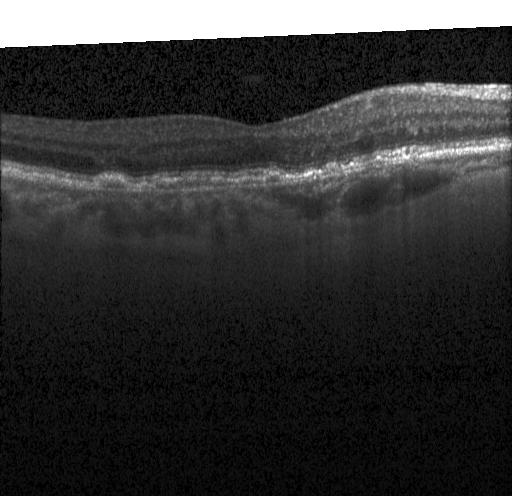 Spectral-domain OCT B-scan: choroidal neovascularization.